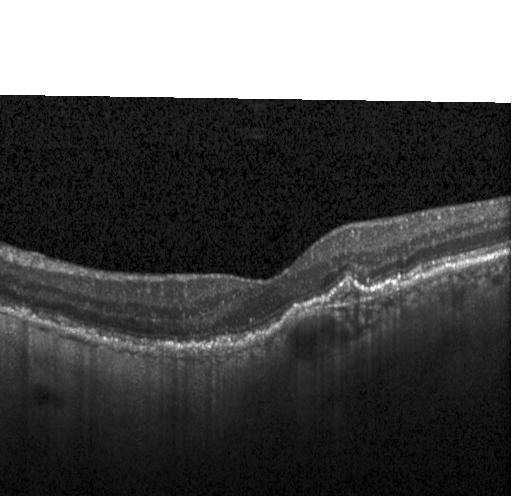
OCT line scan. Instrument: Heidelberg Spectralis. Diagnosis: CNV.